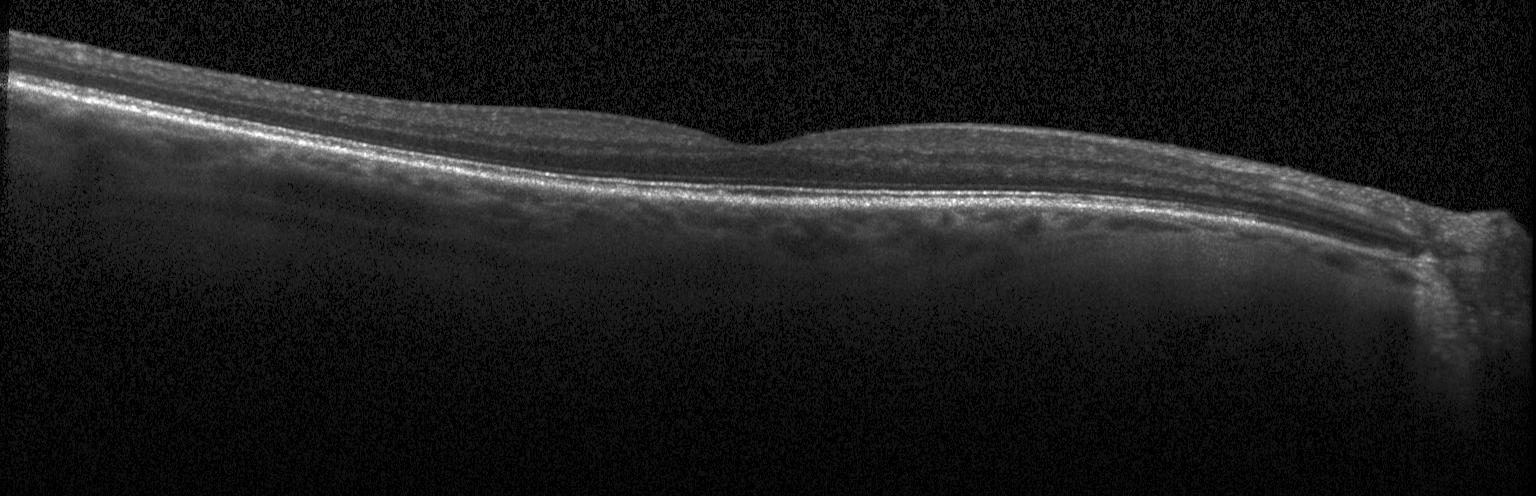

Macular scan; OCT line scan. Impression: no choroidal neovascularization, no diabetic macular edema, and no drusen.